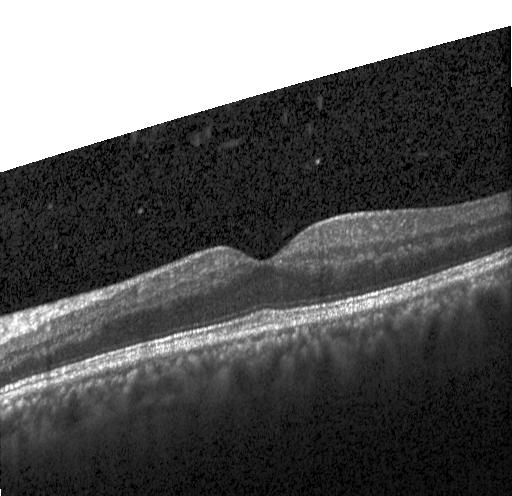

The scan shows no CNV, no DME, and no drusen.